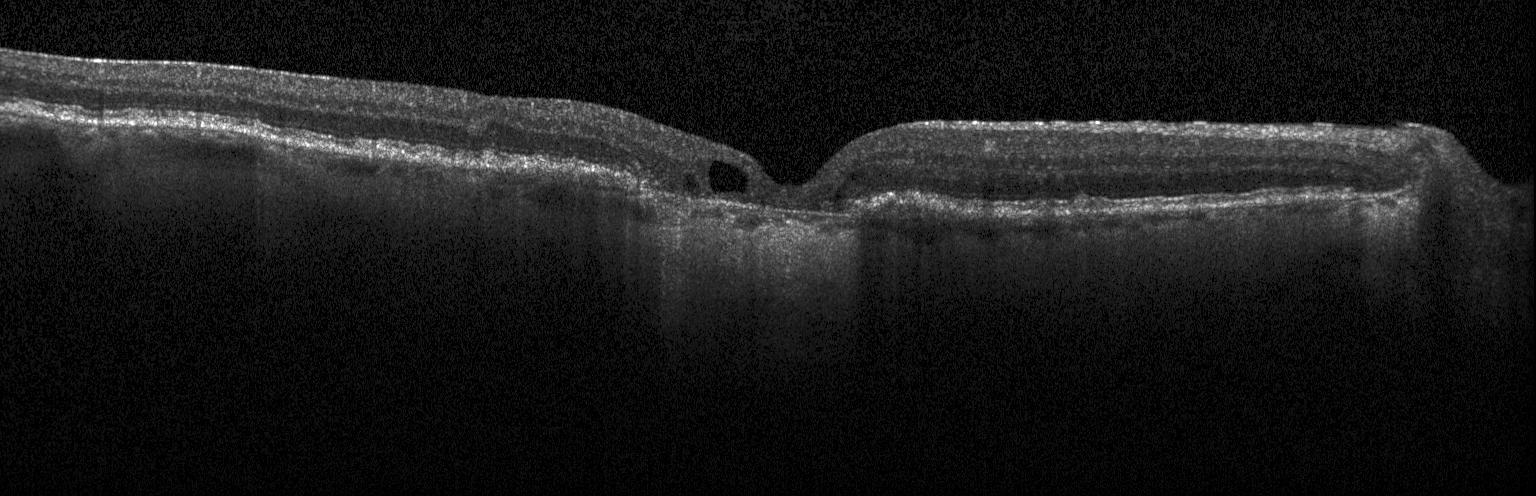 Heidelberg Spectralis OCT system · SD-OCT · through the macula · OCT line scan
Impression: a choroidal neovascular membrane.